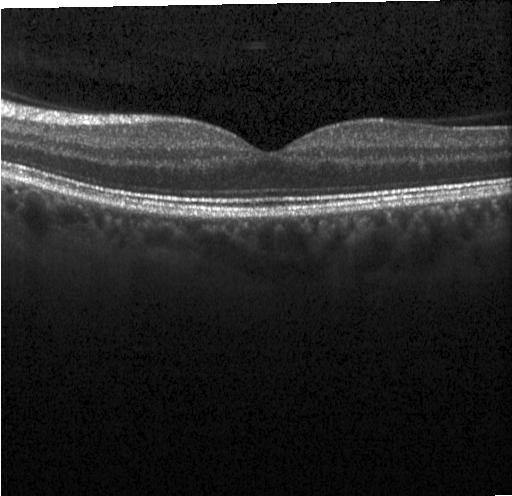 Macular OCT: neither choroidal neovascularization, diabetic macular edema, nor drusen.